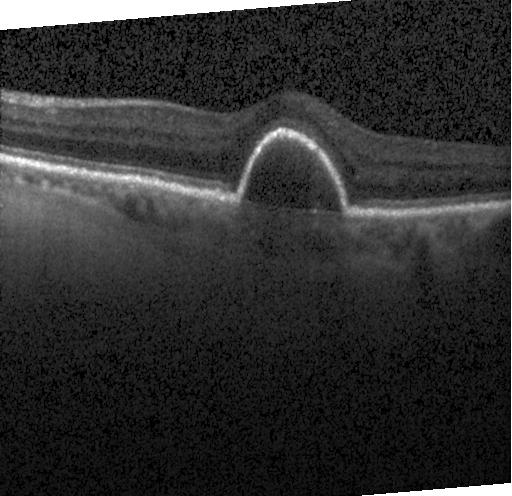
Spectral-domain OCT B-scan: a choroidal neovascular membrane.